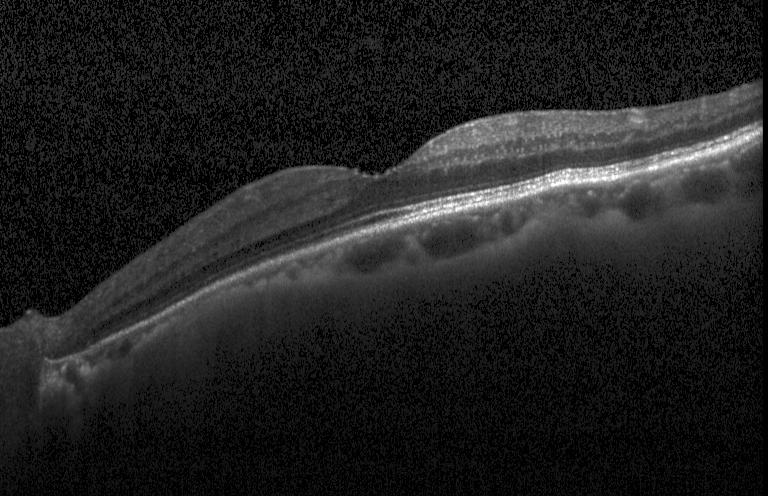

Retinal OCT B-scan; spectral-domain optical coherence tomography; Heidelberg Spectralis; horizontal scan through the fovea.
The scan shows no choroidal neovascularization, diabetic macular edema, or drusen.